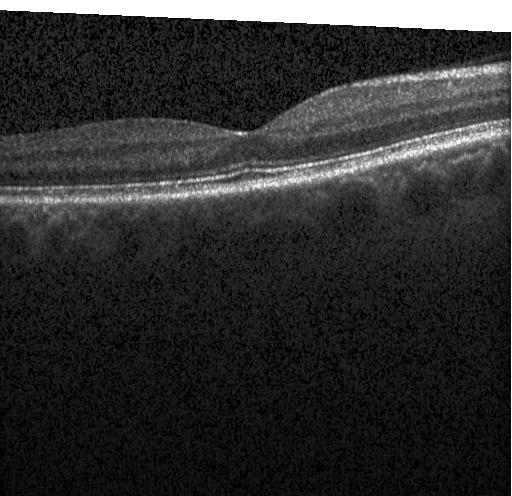 Spectral-domain OCT B-scan: no evidence of choroidal neovascularization, diabetic macular edema, or drusen.